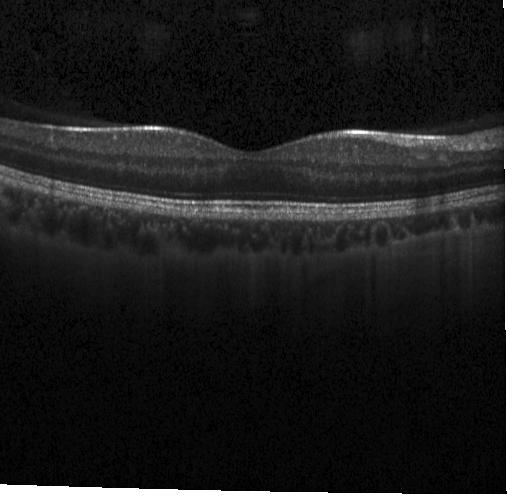 OCT B-scan. Spectral-domain optical coherence tomography. Instrument: Heidelberg Spectralis.
Assessment: no choroidal neovascularization, no diabetic macular edema, and no drusen.